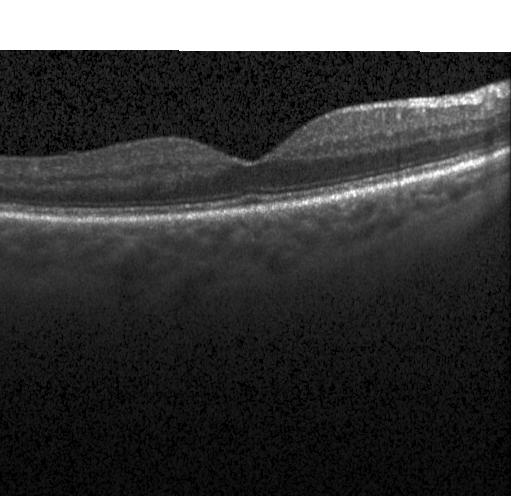 The scan shows no evidence of CNV, DME, or drusen.